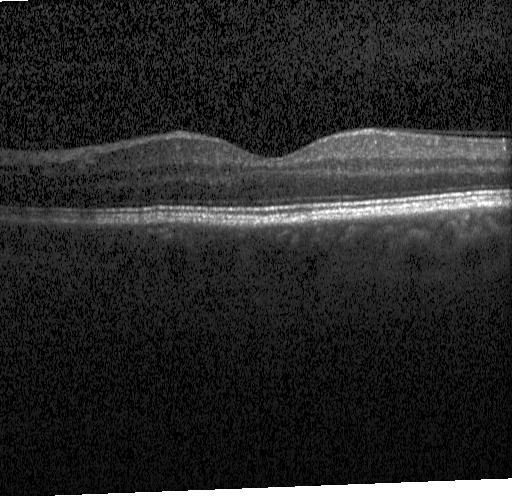

Spectral-domain OCT · Heidelberg Spectralis OCT system · OCT line scan
Assessment: no choroidal neovascularization, no diabetic macular edema, and no drusen.